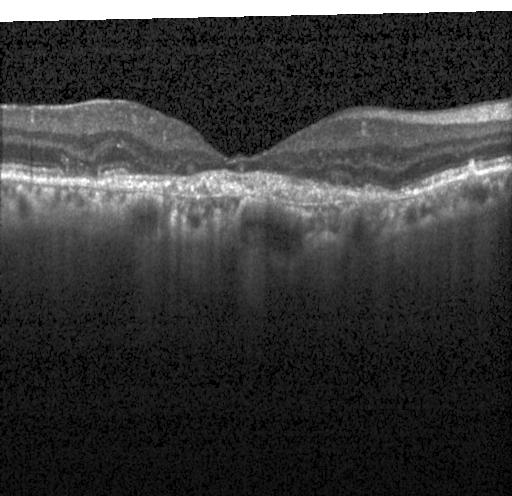

Optical coherence tomography scan. Spectral-domain OCT. Macular scan. A choroidal neovascular membrane.